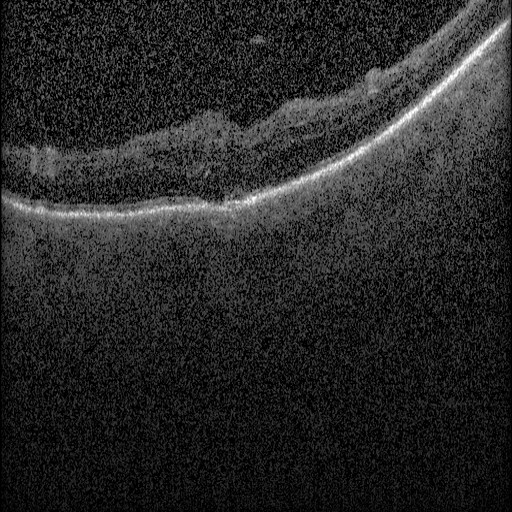

OCT B-scan · SD-OCT.
The scan shows diabetic macular edema (DME).